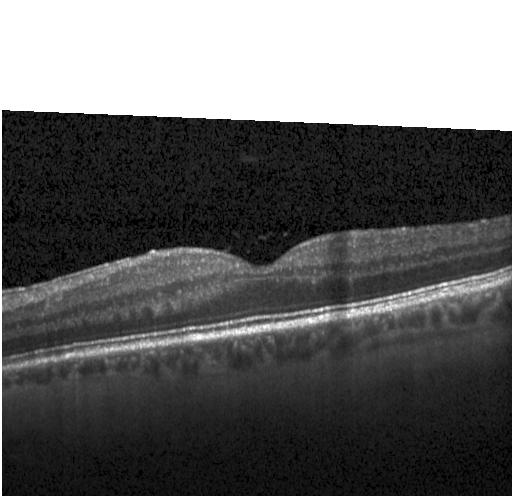

Instrument: Heidelberg Spectralis; OCT line scan; spectral-domain optical coherence tomography; horizontal scan through the fovea
Macular OCT: no CNV, DME, or drusen.